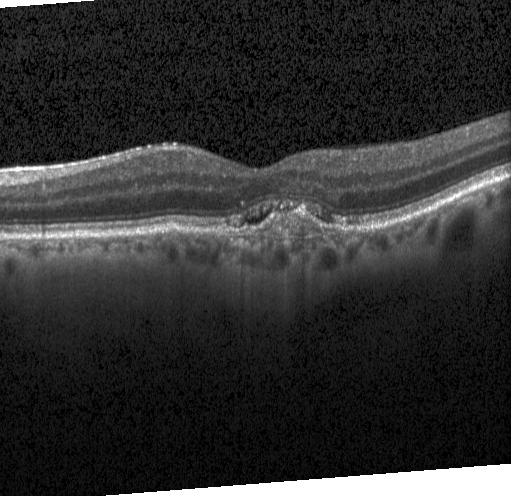

Retinal OCT cross-section; spectral-domain OCT; macular scan — Dx: choroidal neovascularization.